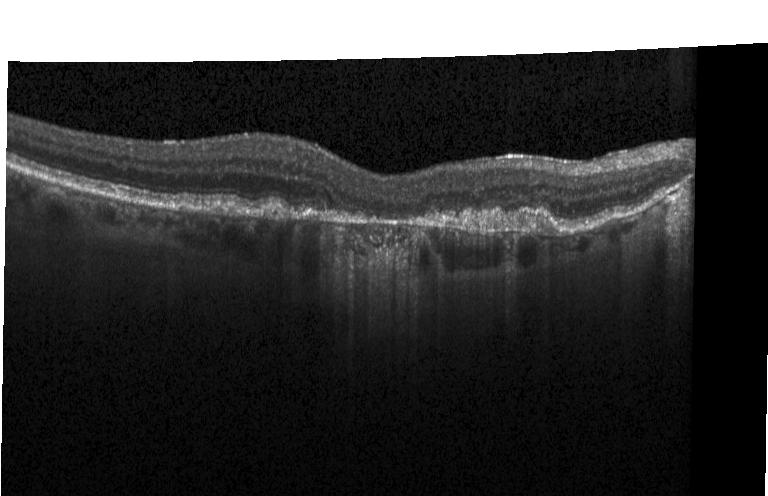 Acquired on a Heidelberg Spectralis, fovea-centered, OCT line scan
Dx: a choroidal neovascular membrane.